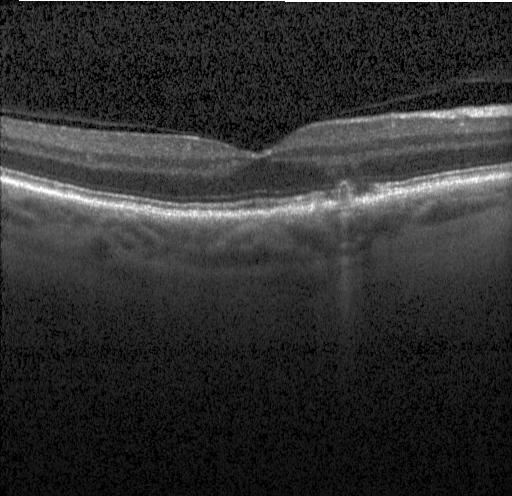 Instrument: Heidelberg Spectralis · spectral-domain OCT · OCT B-scan
Diagnosis: sub-RPE drusenoid deposits.